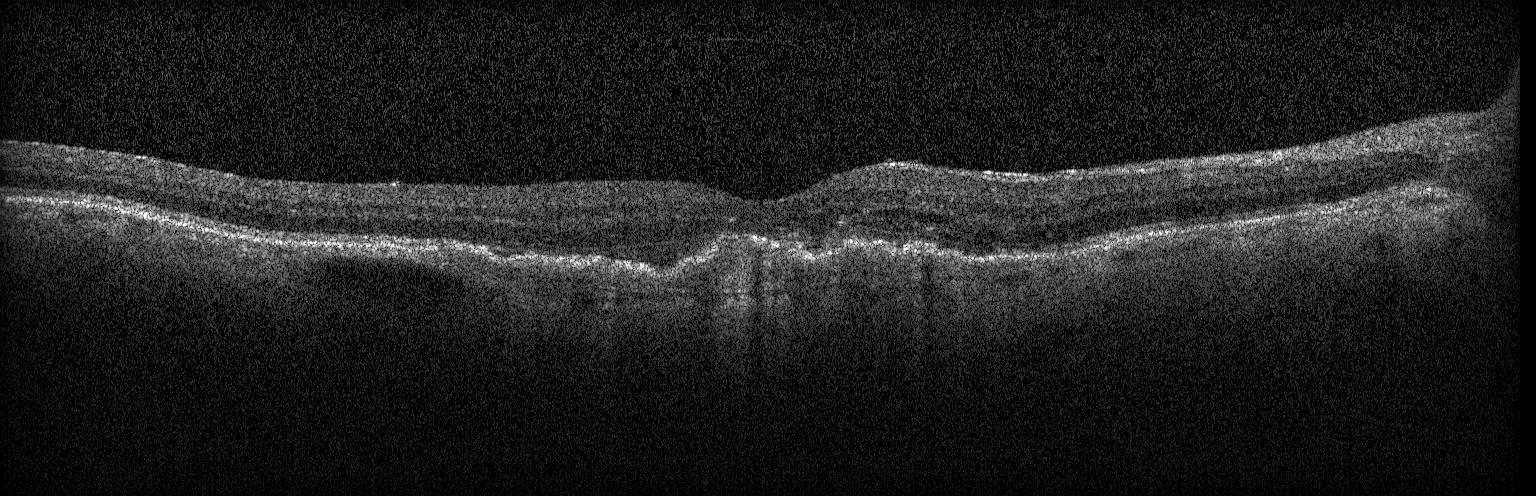
Macular scan. OCT line scan.
OCT finding: a choroidal neovascular membrane.